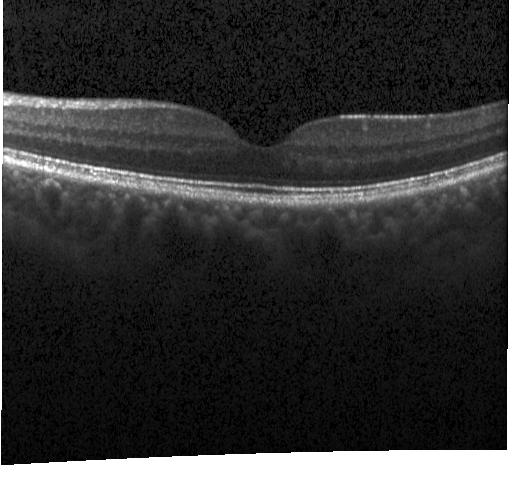

SD-OCT · Heidelberg Spectralis · optical coherence tomography B-scan
No evidence of choroidal neovascularization, diabetic macular edema, or drusen.